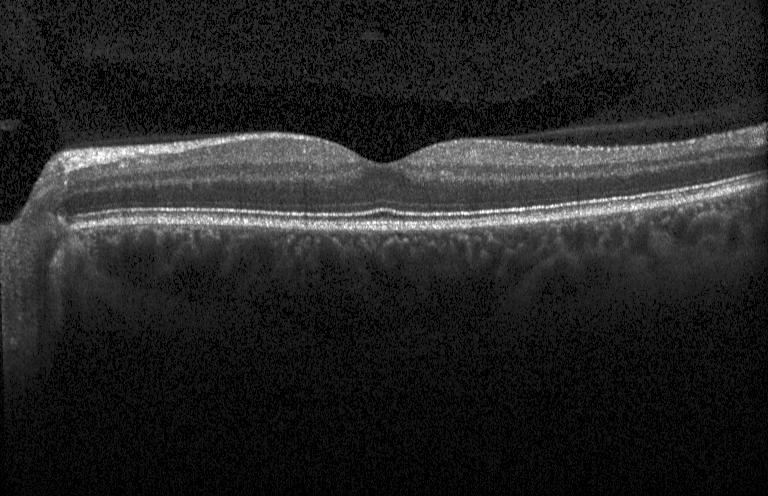 OCT B-scan. Finding: no CNV, no DME, and no drusen.